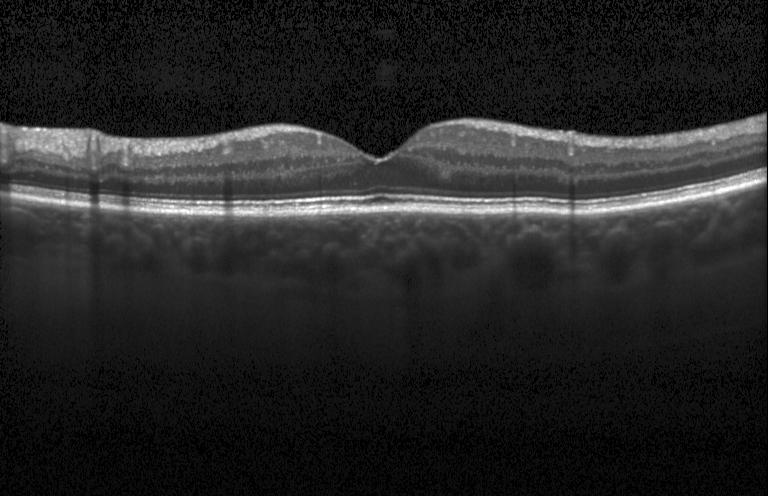 Optical coherence tomography scan. Spectral-domain optical coherence tomography — Diagnosis: no choroidal neovascularization, diabetic macular edema, or drusen.